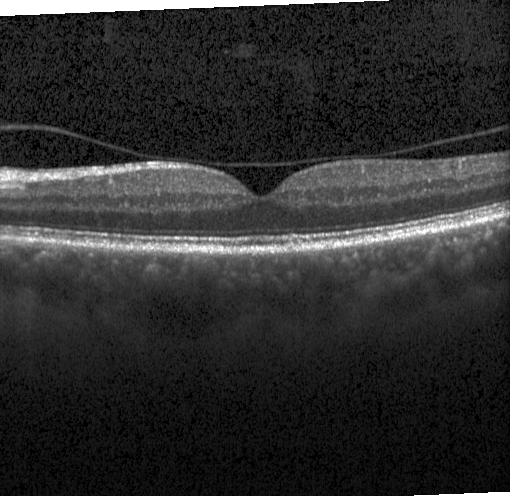

OCT line scan.
OCT finding: no choroidal neovascularization, no diabetic macular edema, and no drusen.